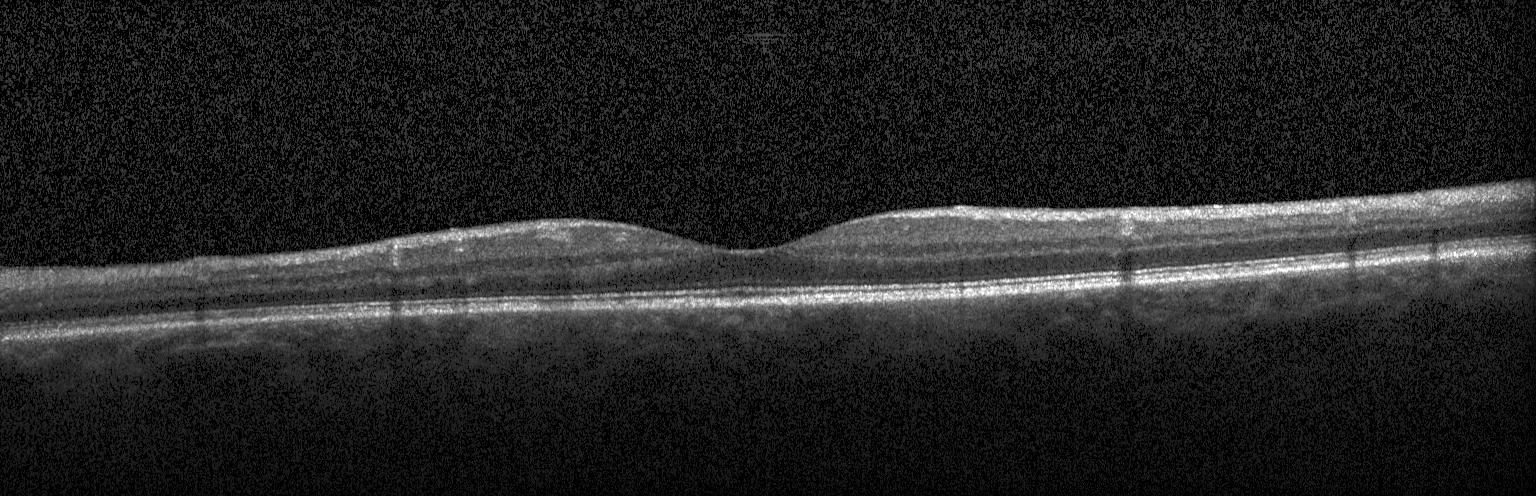

Finding: no choroidal neovascularization, no diabetic macular edema, and no drusen.